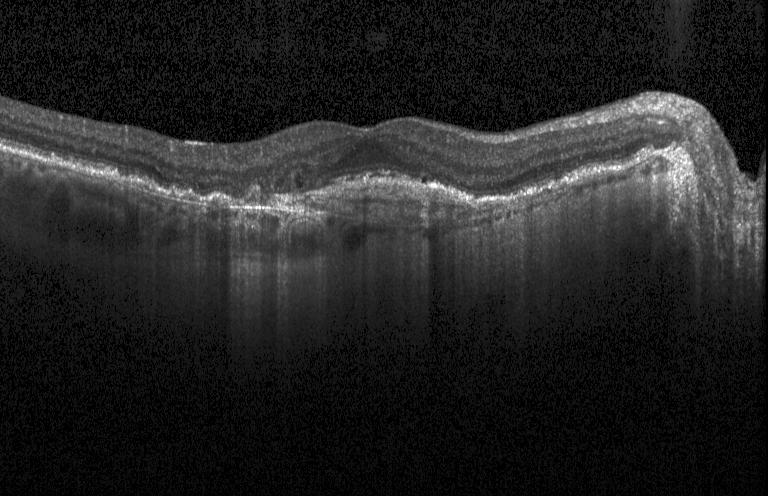

Finding: a choroidal neovascular membrane.